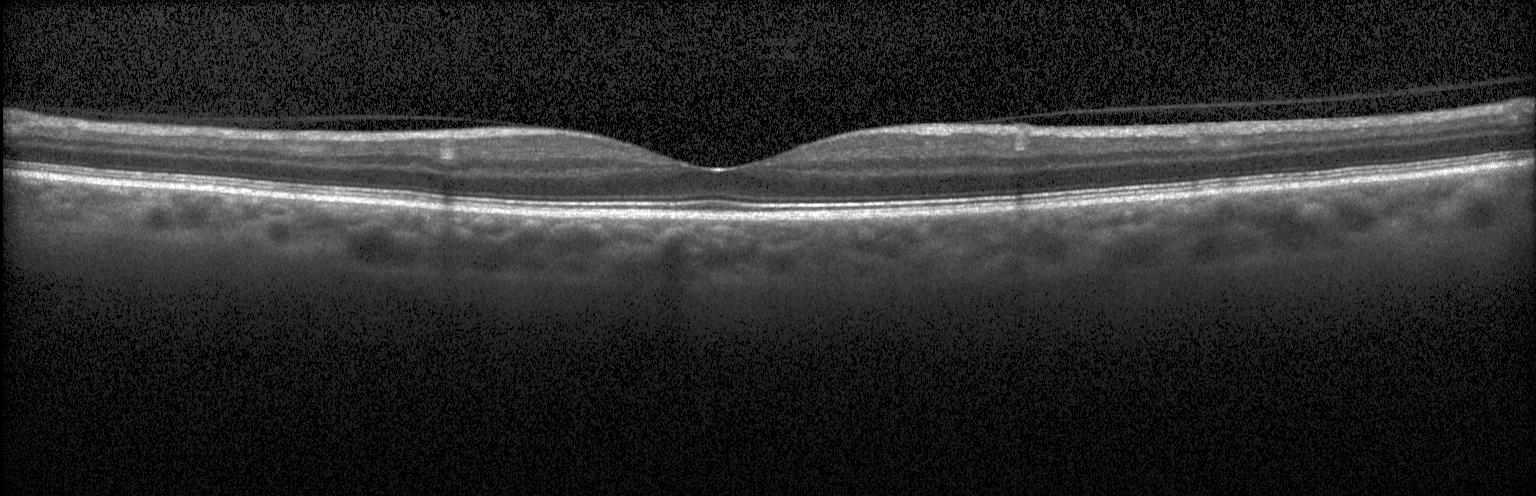 OCT B-scan. This B-scan demonstrates no evidence of choroidal neovascularization, diabetic macular edema, or drusen.